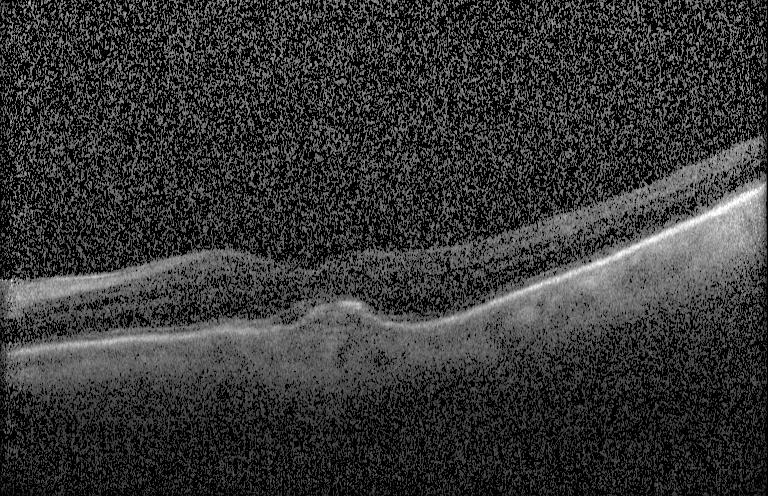 Horizontal scan through the fovea · spectral-domain OCT · retinal OCT B-scan · instrument: Heidelberg Spectralis — OCT finding: a choroidal neovascular membrane.